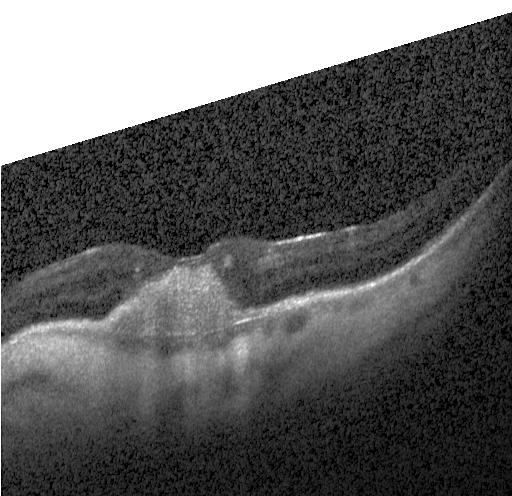
Retinal OCT B-scan
Diagnosis: CNV.